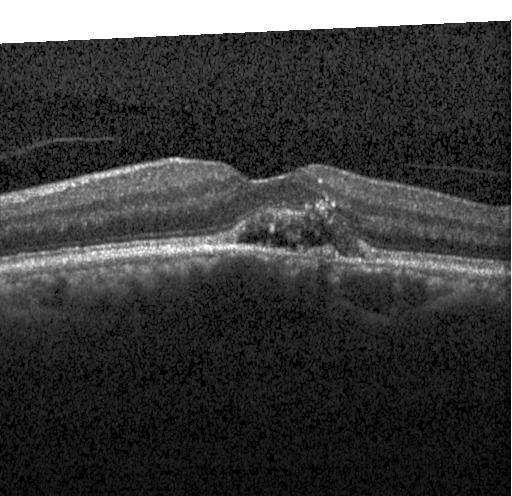

Finding: a choroidal neovascular membrane.